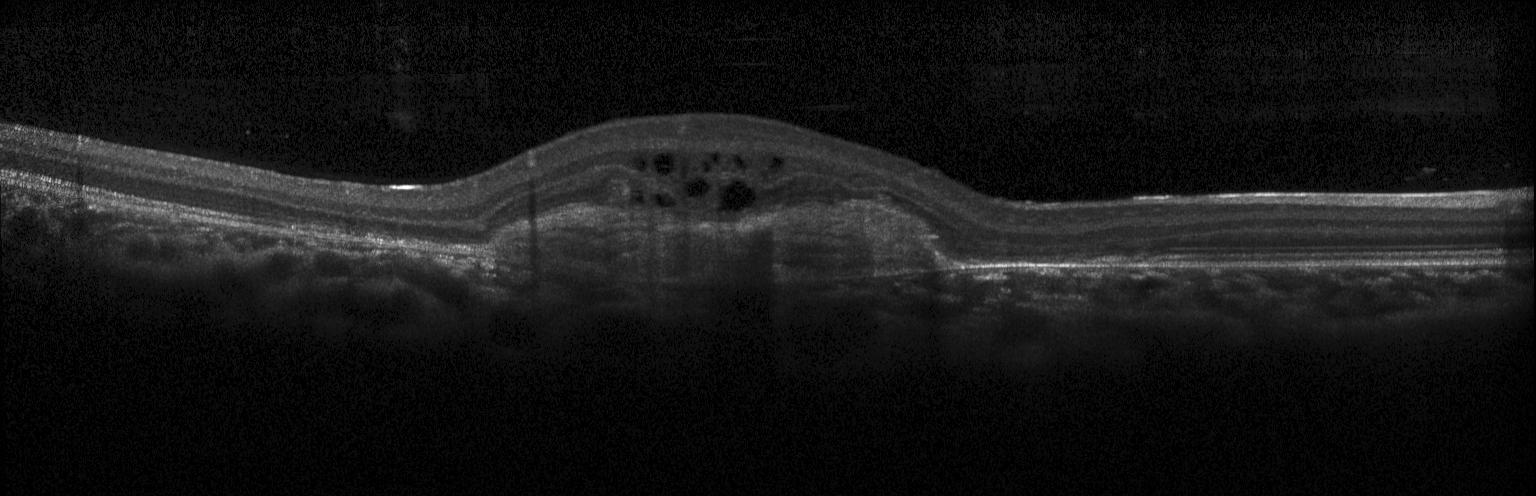
Optical coherence tomography B-scan; macular scan — CNV.